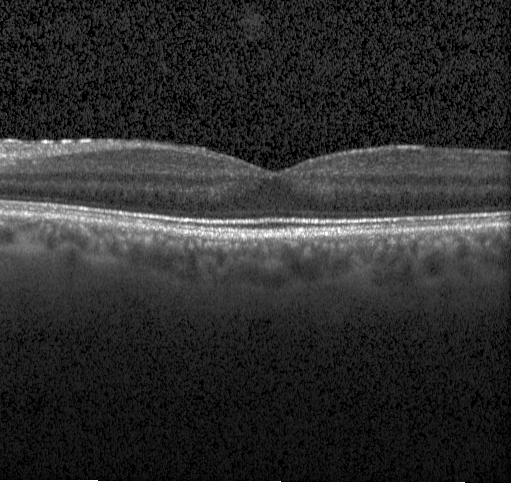

OCT B-scan, through the macula, SD-OCT — This B-scan demonstrates neither choroidal neovascularization, diabetic macular edema, nor drusen.